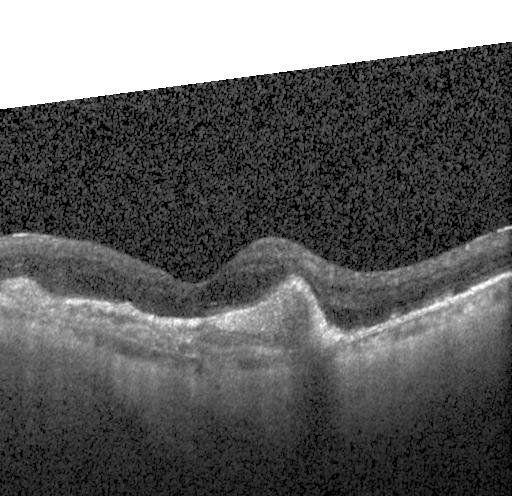
Heidelberg Spectralis · through the macula · OCT line scan. OCT finding: a choroidal neovascular membrane.